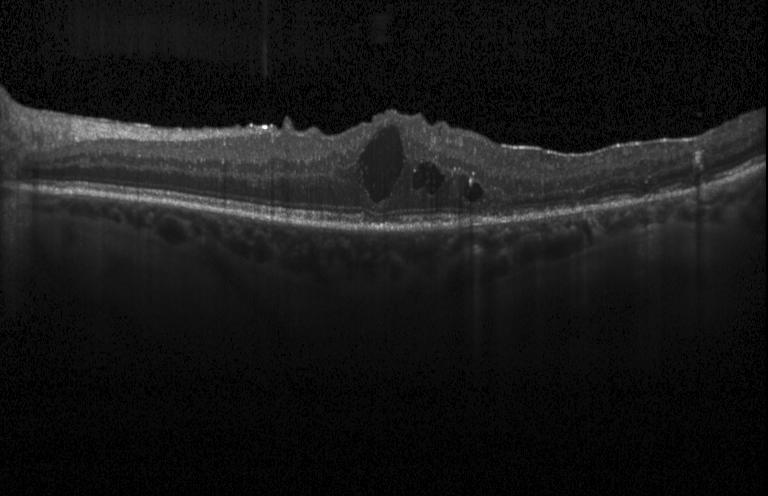 Optical coherence tomography scan; horizontal scan through the fovea; Heidelberg Spectralis; spectral-domain OCT — Dx: diabetic macular edema (DME).